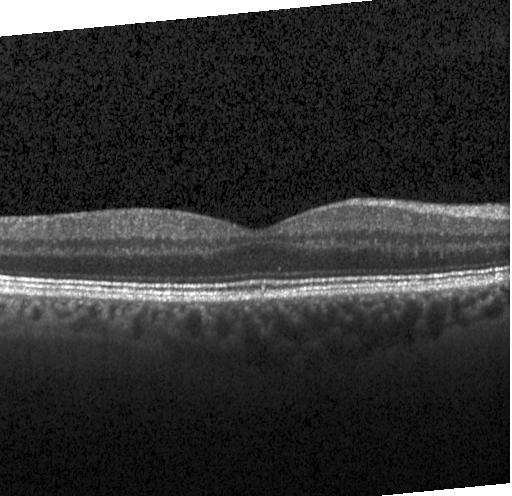
Heidelberg Spectralis OCT system, spectral-domain OCT, optical coherence tomography B-scan
Finding: neither choroidal neovascularization, diabetic macular edema, nor drusen.